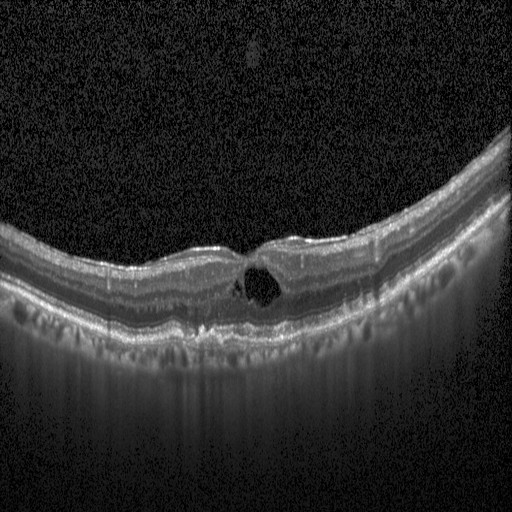 OCT line scan, fovea-centered, Heidelberg Spectralis OCT system. Impression: diabetic macular edema (DME).